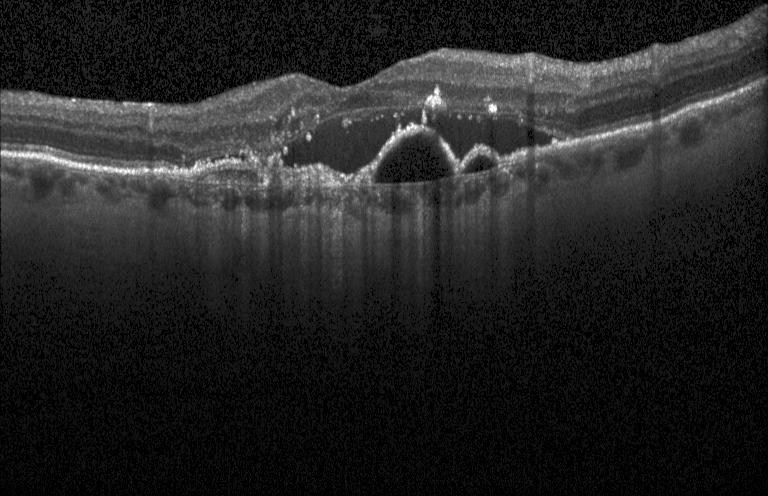 Heidelberg Spectralis. Optical coherence tomography B-scan. Spectral-domain OCT — This B-scan demonstrates a choroidal neovascular membrane.